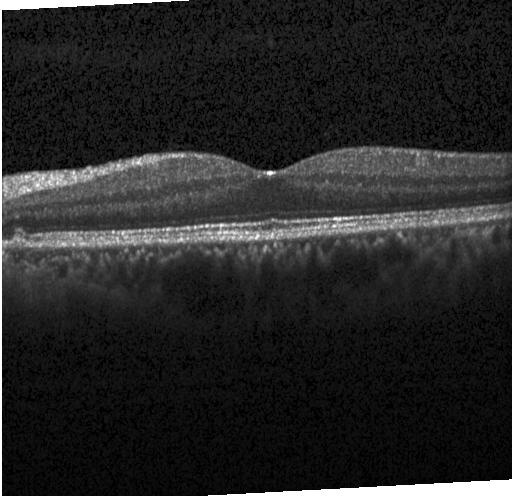

OCT line scan; spectral-domain OCT; horizontal scan through the fovea; Heidelberg Spectralis
Macular OCT: no CNV, no DME, and no drusen.